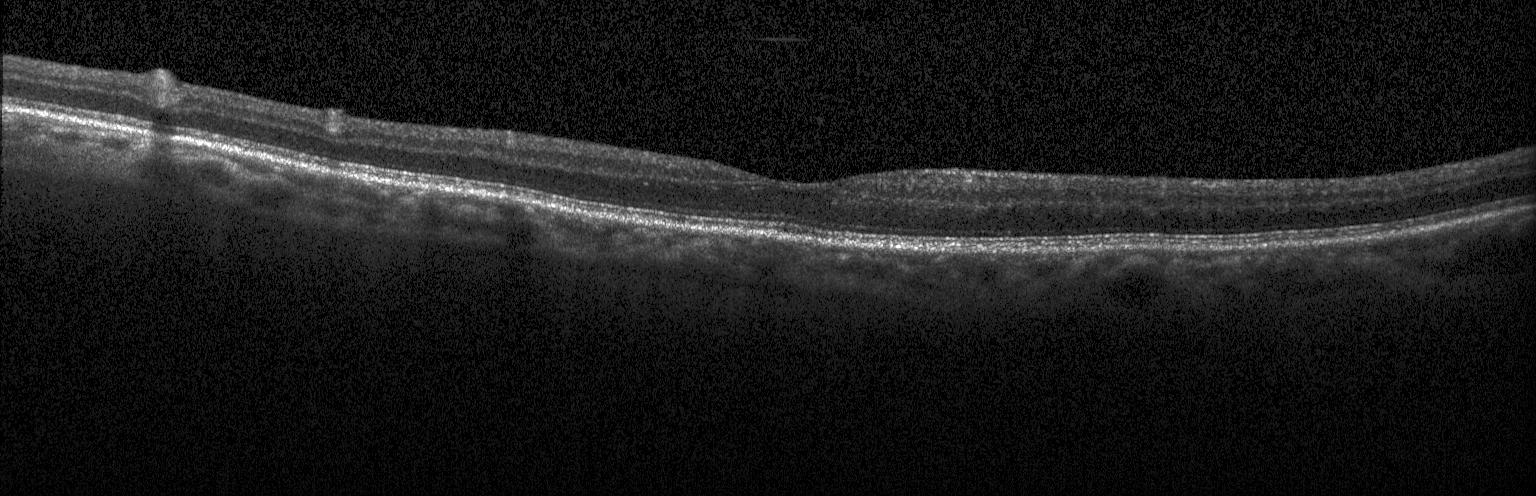 Acquired on a Heidelberg Spectralis; horizontal scan through the fovea; optical coherence tomography B-scan. Impression: no CNV, no DME, and no drusen.